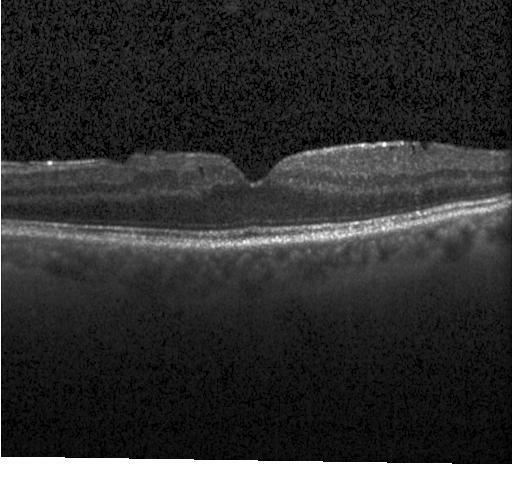
OCT line scan; fovea-centered; acquired on a Heidelberg Spectralis; spectral-domain optical coherence tomography.
The scan shows DME.